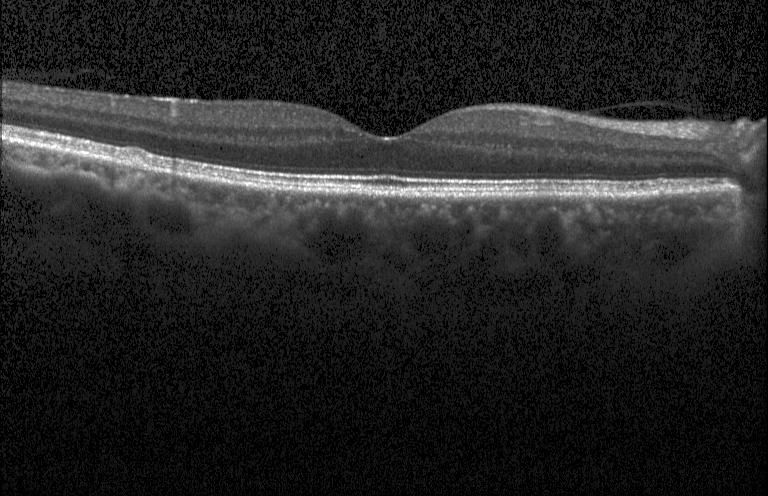
Retinal OCT B-scan
Dx: neither CNV, DME, nor drusen.